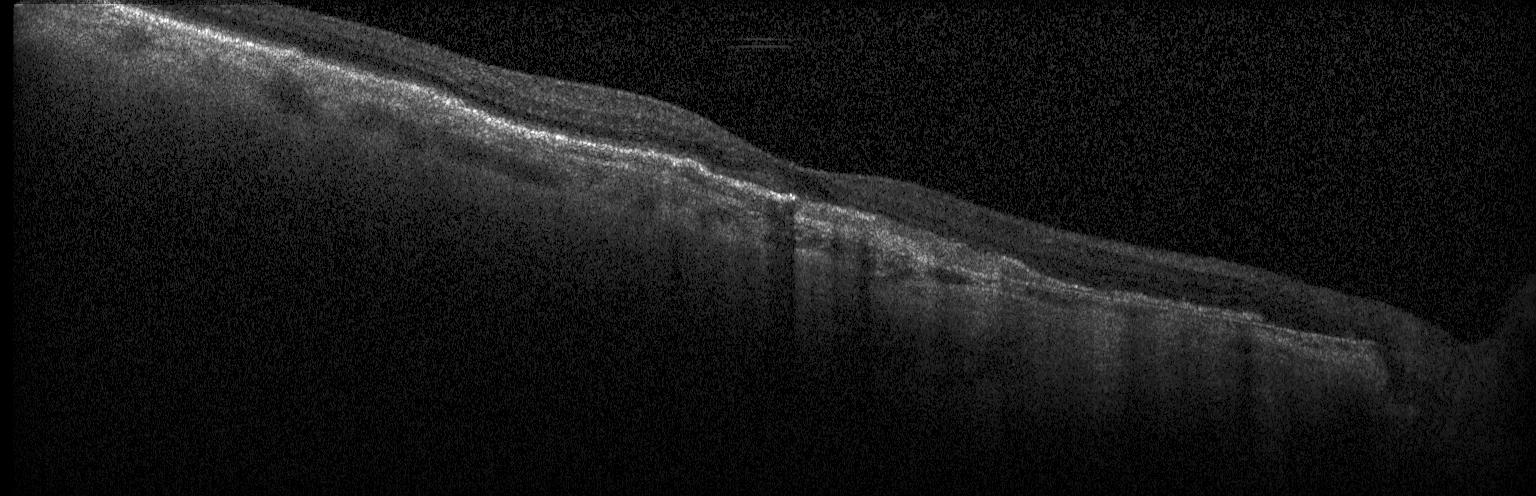 Retinal OCT B-scan
Impression: CNV.